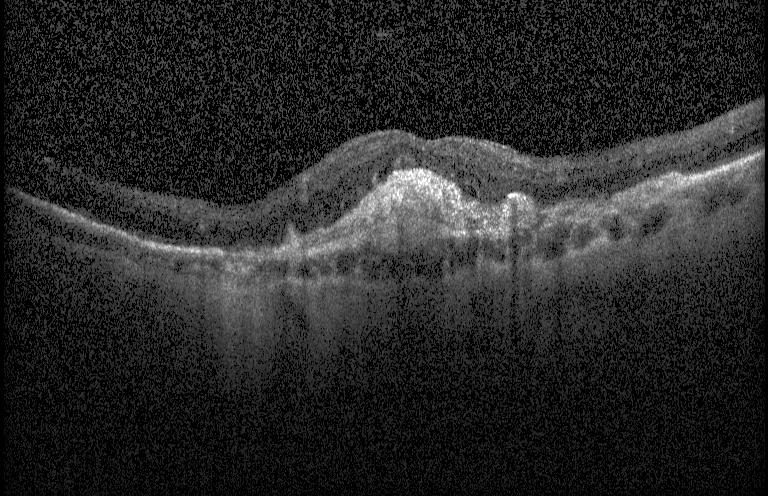 OCT B-scan showing a choroidal neovascular membrane.